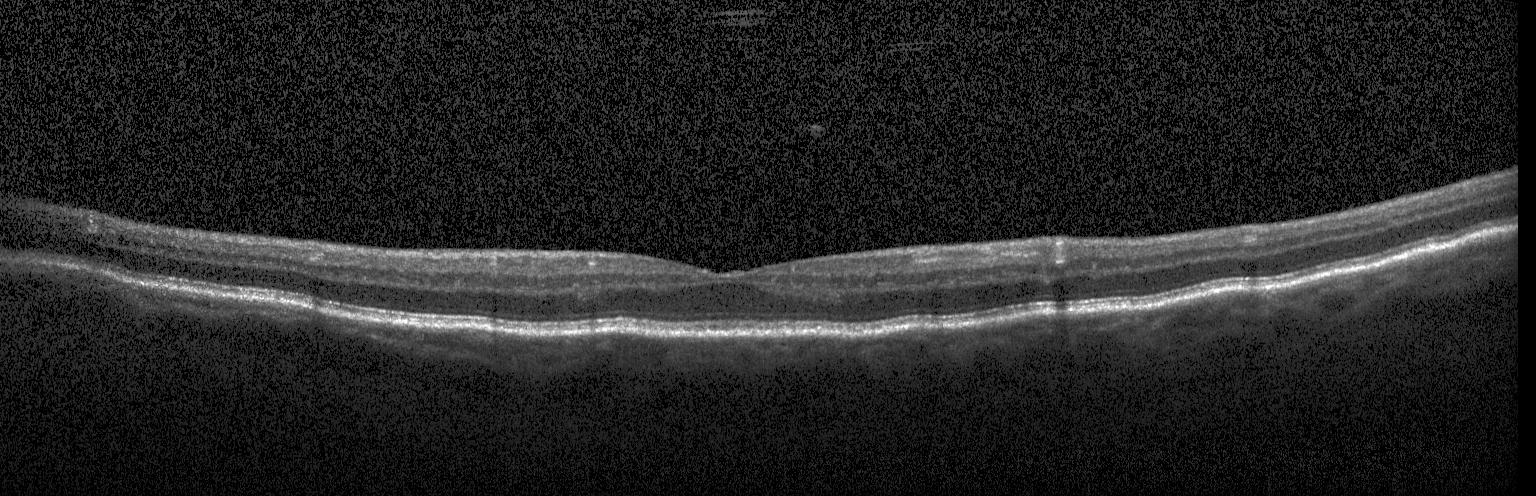 Optical coherence tomography scan · Heidelberg Spectralis OCT system · spectral-domain optical coherence tomography · macular scan. This B-scan demonstrates no choroidal neovascularization, no diabetic macular edema, and no drusen.